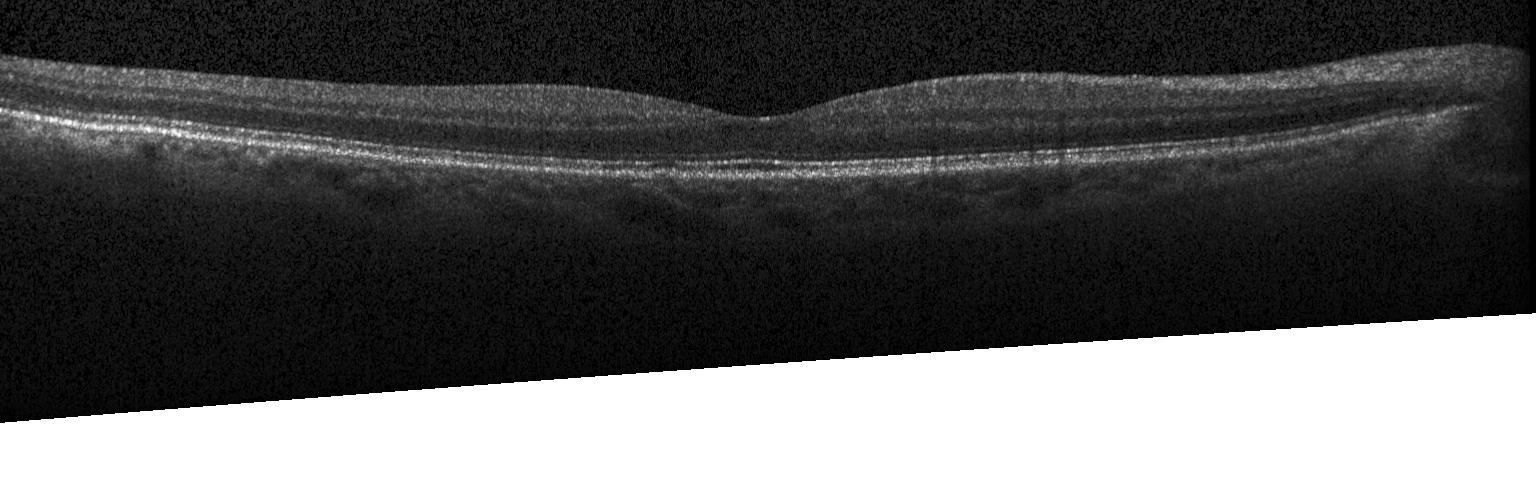
Spectral-domain optical coherence tomography · acquired on a Heidelberg Spectralis · optical coherence tomography scan · macular scan
Finding: no choroidal neovascularization, no diabetic macular edema, and no drusen.